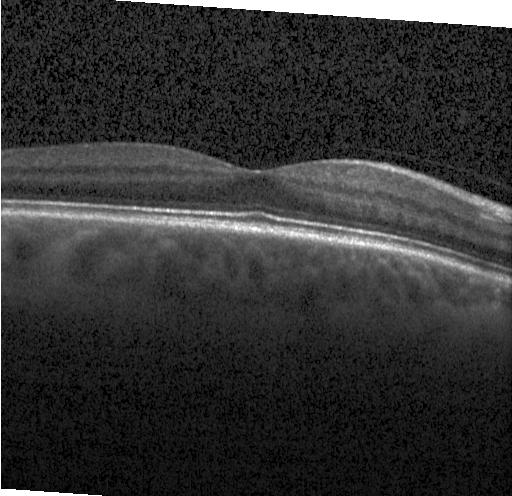 Dx: no choroidal neovascularization, no diabetic macular edema, and no drusen.